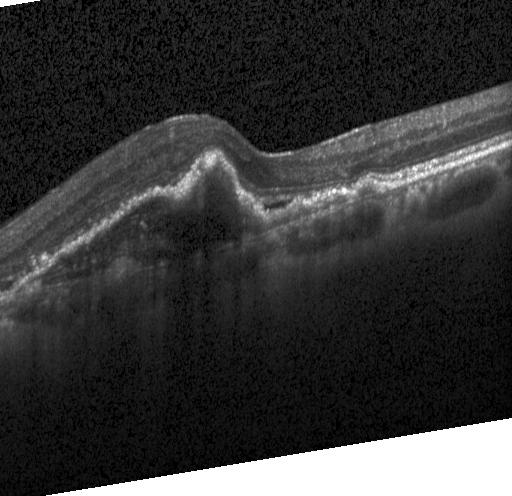

OCT line scan.
Impression: choroidal neovascularization (CNV).